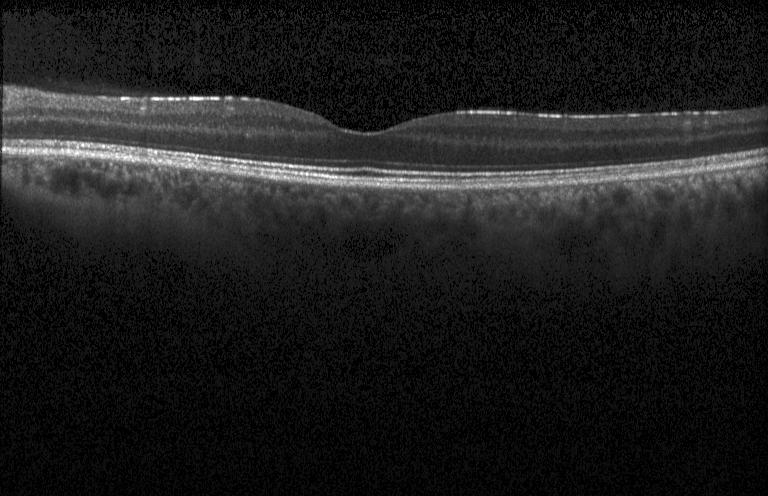 Fovea-centered, SD-OCT, OCT B-scan.
No CNV, DME, or drusen.